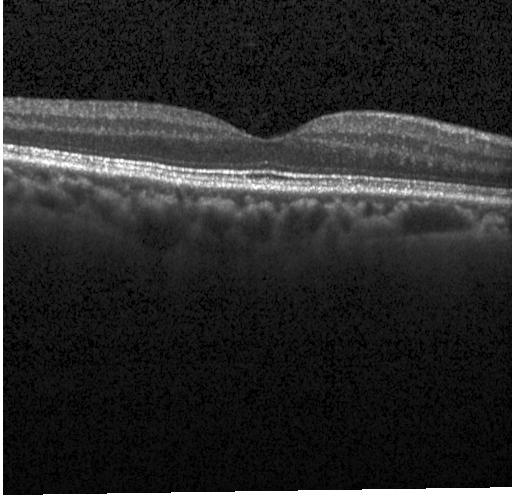
Centered on the fovea. OCT line scan. SD-OCT. Heidelberg Spectralis.
OCT finding: no choroidal neovascularization, no diabetic macular edema, and no drusen.